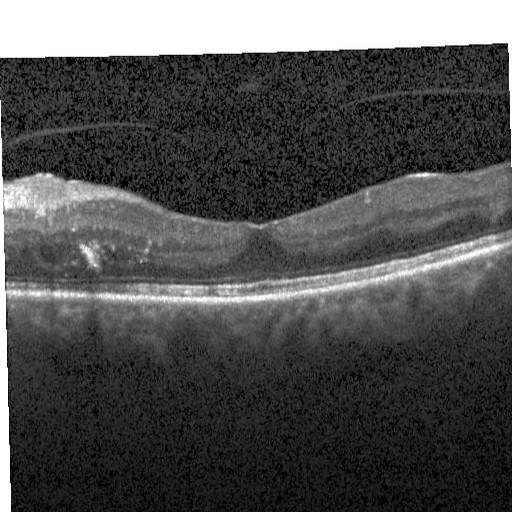

OCT B-scan · spectral-domain OCT — Finding: diabetic macular edema (DME).